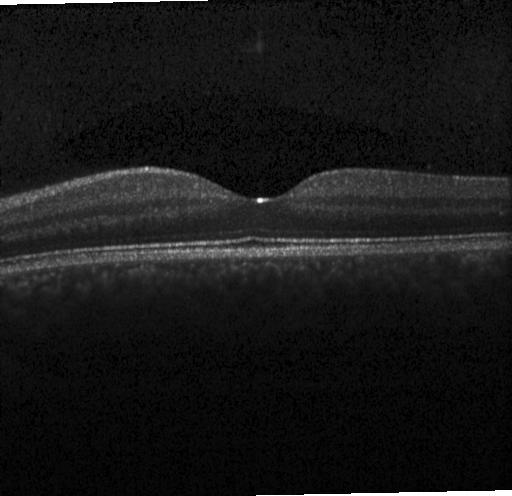 Retinal OCT B-scan.
Impression: no choroidal neovascularization, no diabetic macular edema, and no drusen.